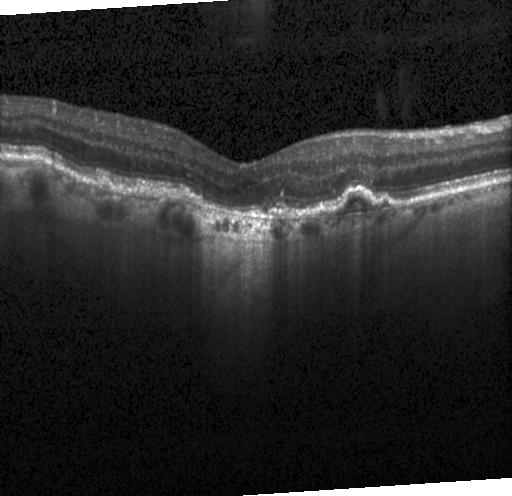

Retinal OCT cross-section. Heidelberg Spectralis. Impression: a choroidal neovascular membrane.